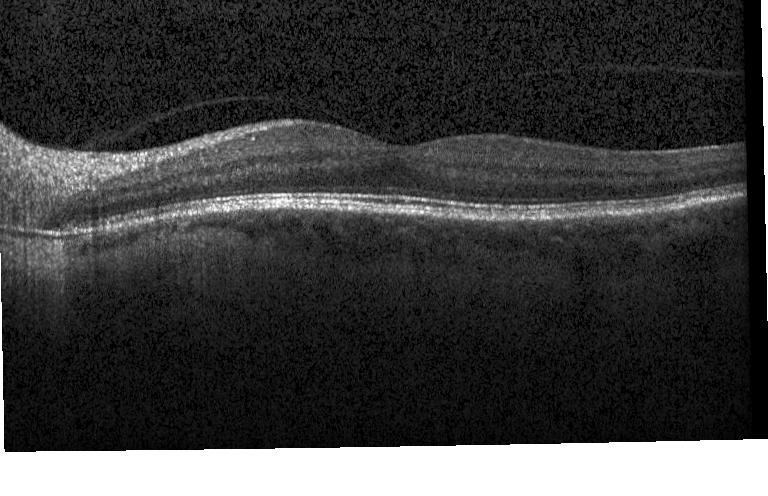 Impression: no choroidal neovascularization, no diabetic macular edema, and no drusen.